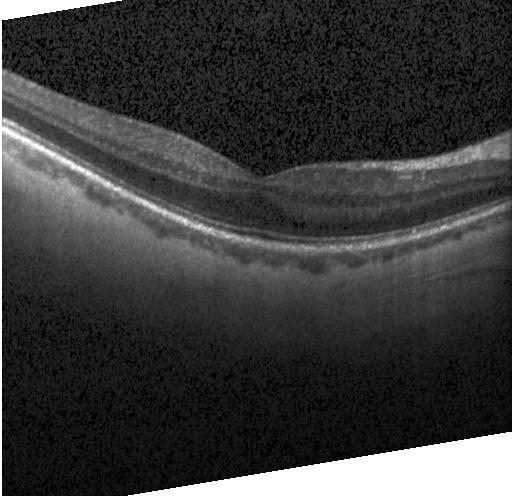

Optical coherence tomography B-scan · SD-OCT · fovea-centered
Impression: no CNV, no DME, and no drusen.